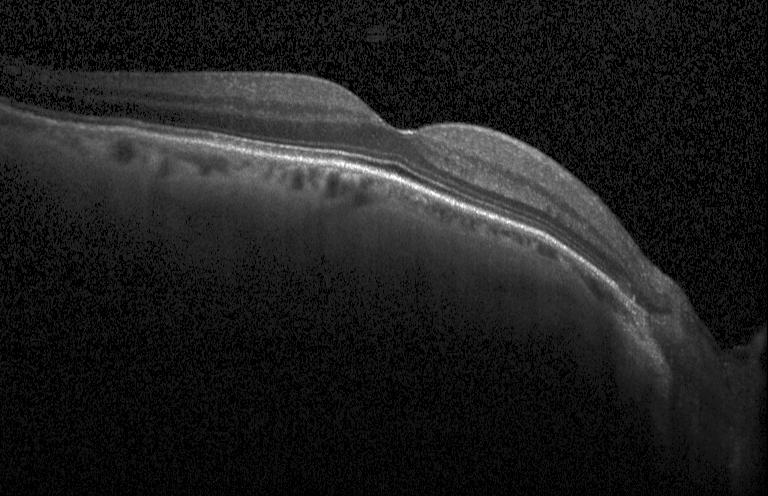
Macular OCT: neither choroidal neovascularization, diabetic macular edema, nor drusen.